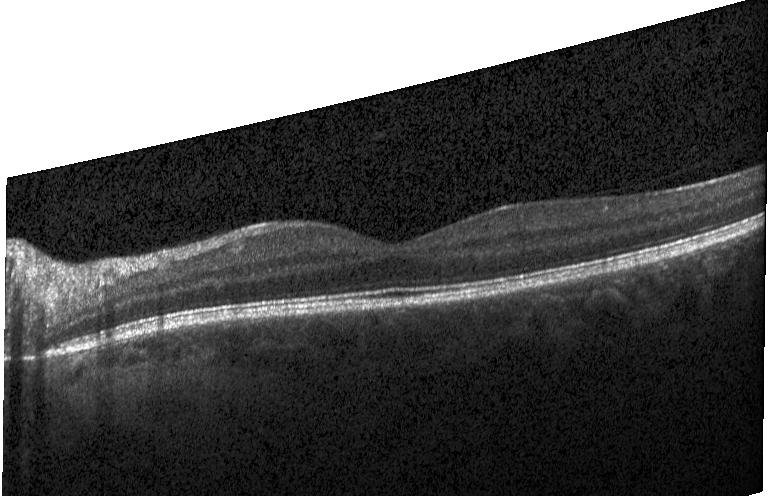

SD-OCT. OCT B-scan. Fovea-centered. Instrument: Heidelberg Spectralis — Diagnosis: no choroidal neovascularization, no diabetic macular edema, and no drusen.